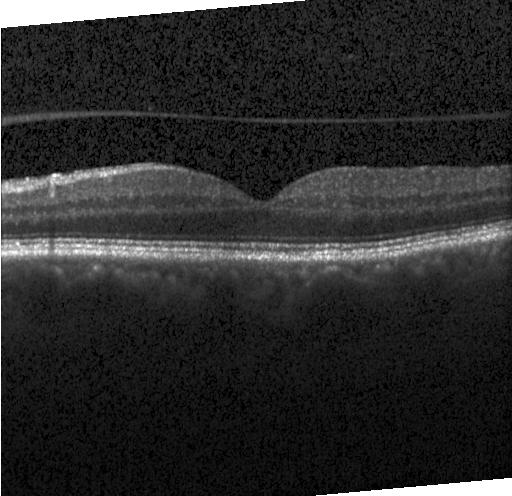
Optical coherence tomography B-scan · acquired on a Heidelberg Spectralis · macular scan · spectral-domain optical coherence tomography — Impression: neither choroidal neovascularization, diabetic macular edema, nor drusen.